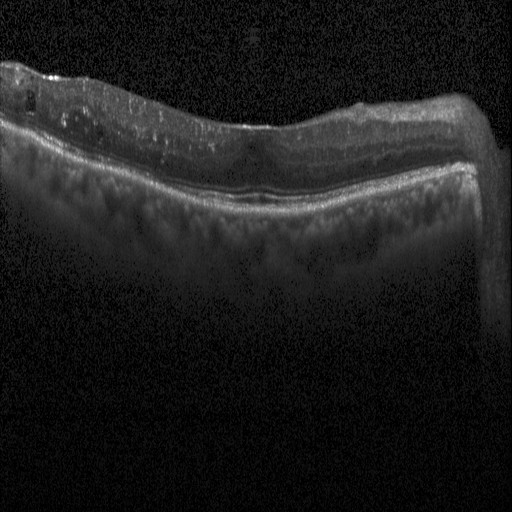 Retinal OCT cross-section
Macular OCT: DME.